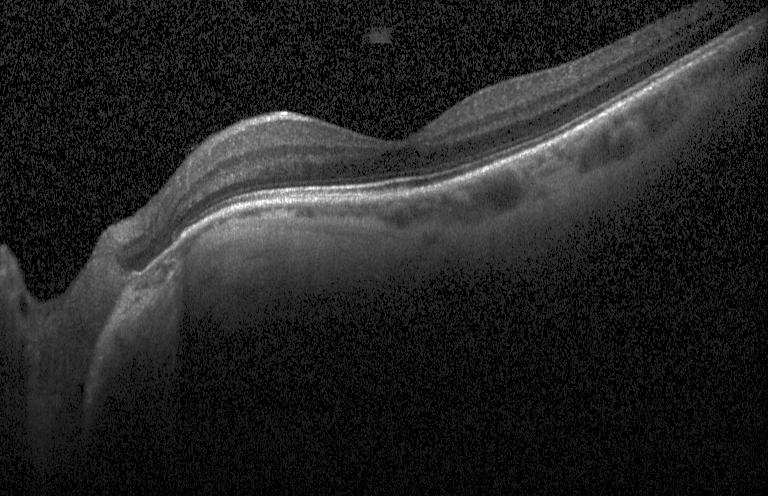 Assessment: no evidence of choroidal neovascularization, diabetic macular edema, or drusen.